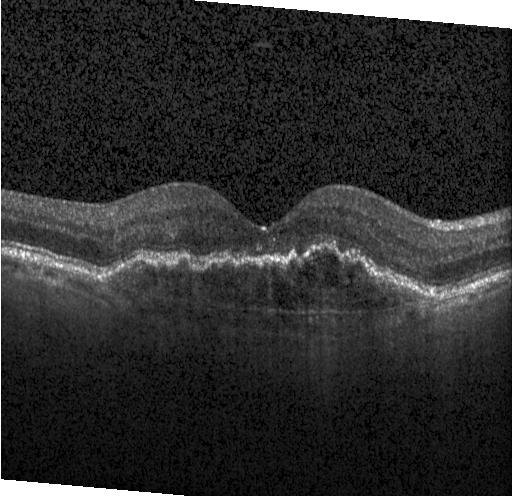
Optical coherence tomography scan, macular scan, spectral-domain OCT.
Finding: a choroidal neovascular membrane.